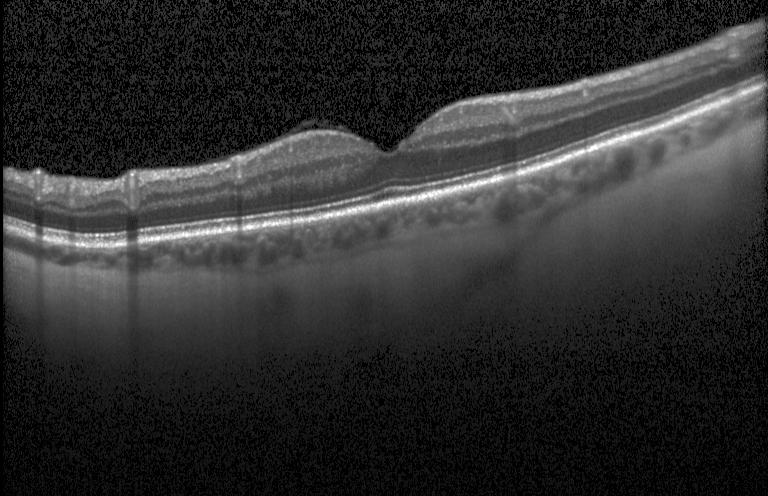
Diagnosis: no CNV, DME, or drusen.